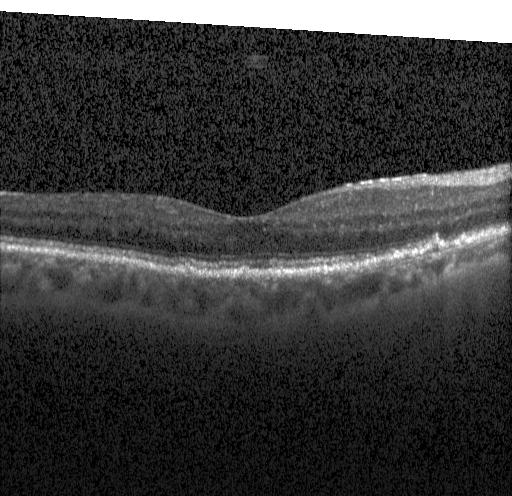

Impression: multiple drusen.